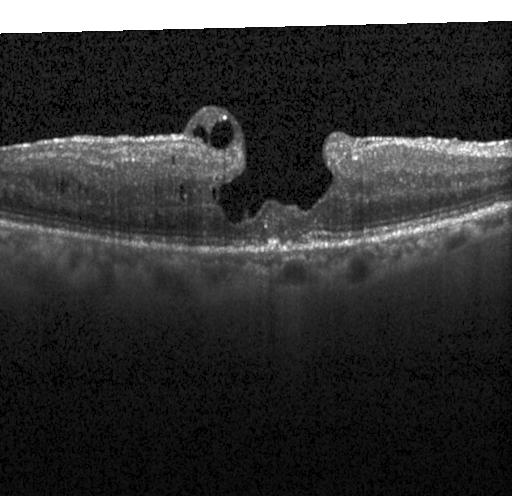

Diagnosis: DME.